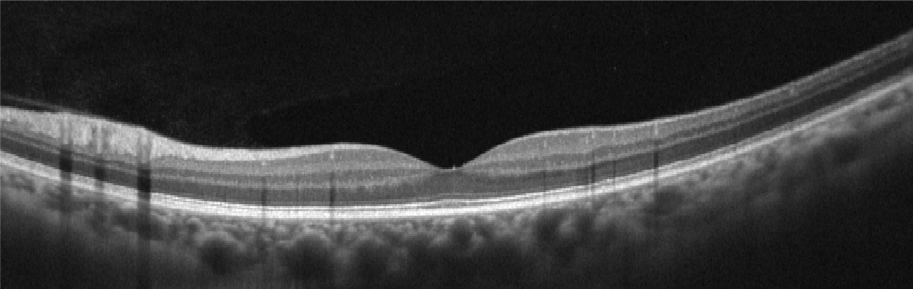
Retinal OCT cross-section showing no AMD, DME, ERM, RAO, RVO, or VID.